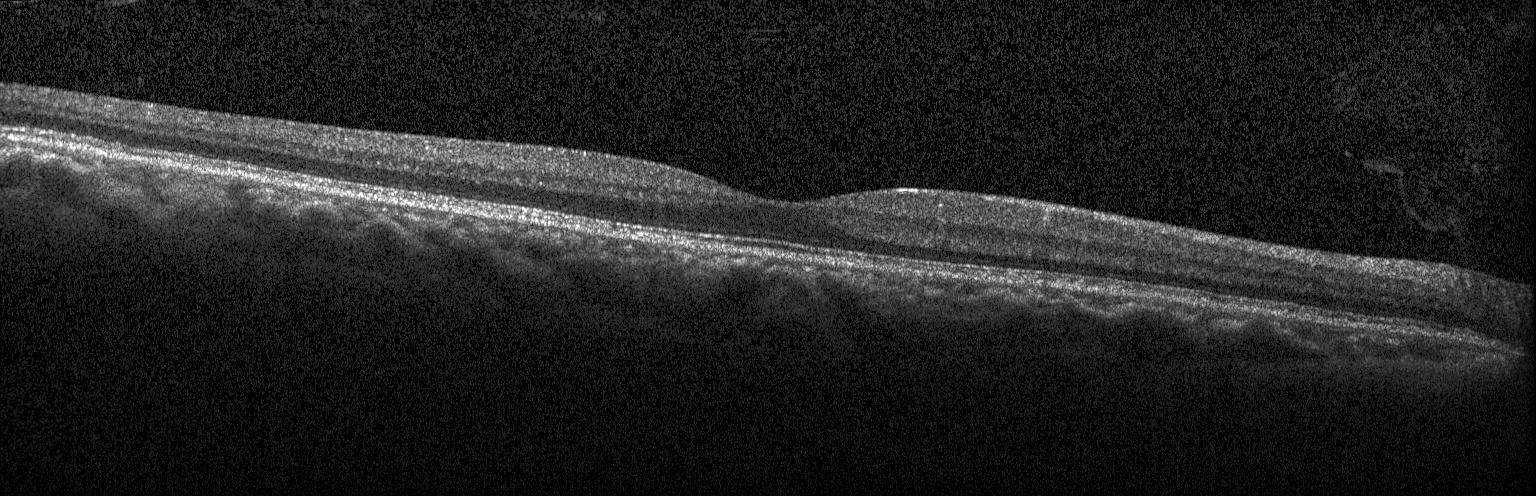

Spectral-domain OCT, Heidelberg Spectralis, centered on the fovea, optical coherence tomography B-scan. Impression: neither CNV, DME, nor drusen.